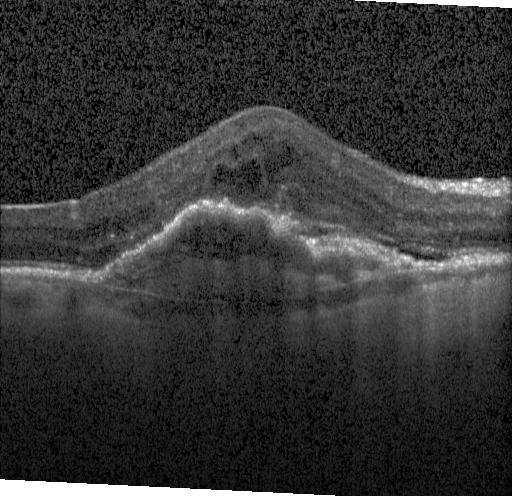
Acquired on a Heidelberg Spectralis, retinal OCT cross-section, horizontal scan through the fovea, SD-OCT. Impression: a choroidal neovascular membrane.